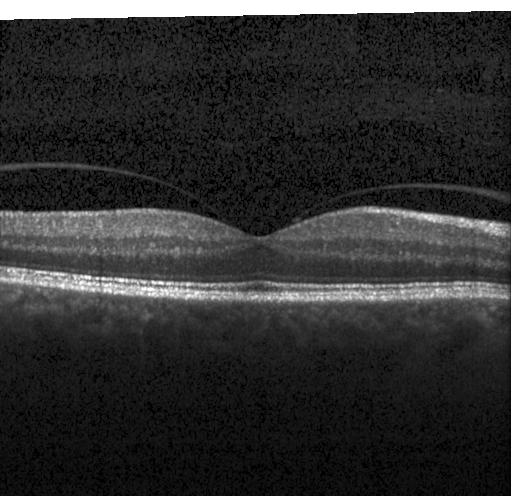

Assessment: no choroidal neovascularization, diabetic macular edema, or drusen.